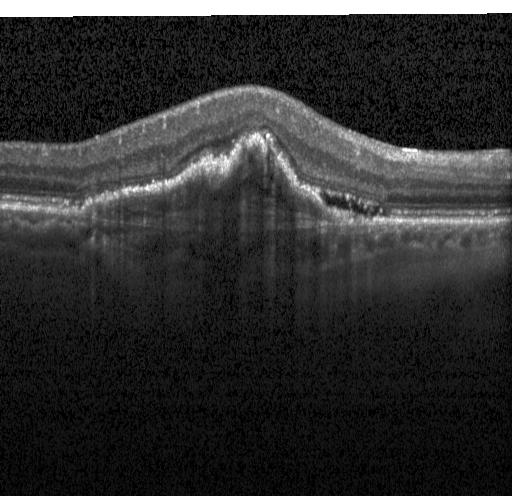 Heidelberg Spectralis OCT system, through the macula, optical coherence tomography scan
Finding: a choroidal neovascular membrane.